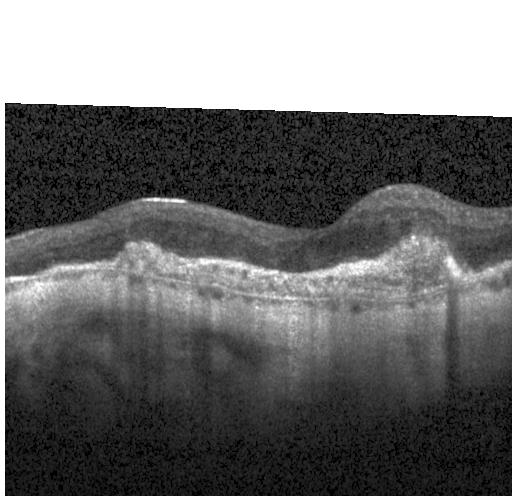 Heidelberg Spectralis; optical coherence tomography B-scan — Finding: a choroidal neovascular membrane.